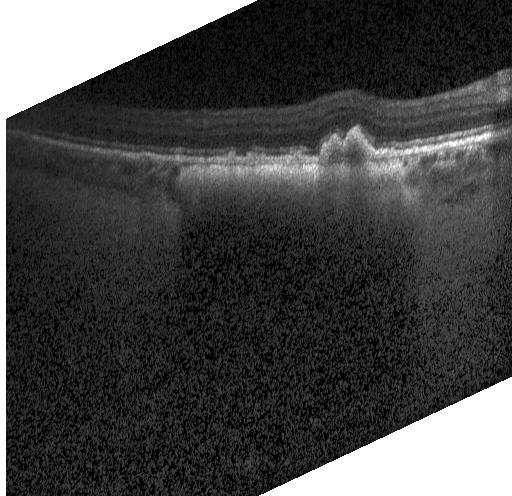

Acquired on a Heidelberg Spectralis. Retinal OCT B-scan. Spectral-domain optical coherence tomography.
OCT finding: a choroidal neovascular membrane.